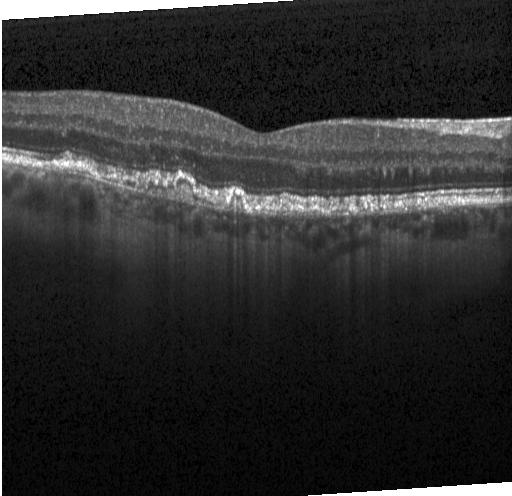
Retinal OCT cross-section; Heidelberg Spectralis OCT system; spectral-domain OCT. Finding: drusen.